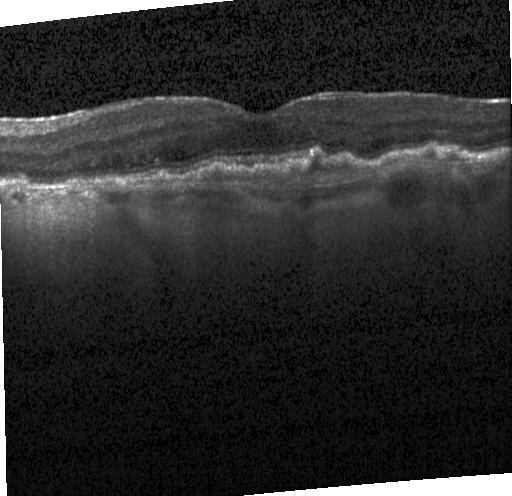
Retinal OCT cross-section showing CNV.